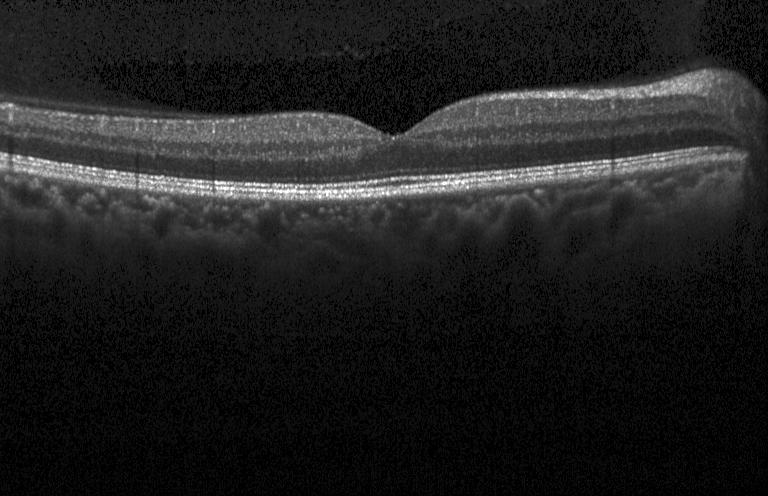 OCT B-scan showing no CNV, no DME, and no drusen.